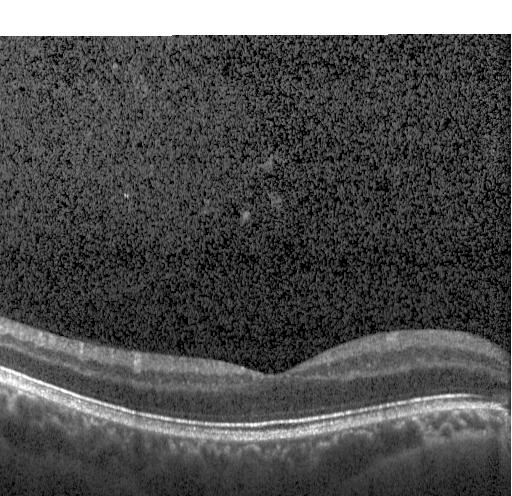 Retinal OCT cross-section showing no evidence of choroidal neovascularization, diabetic macular edema, or drusen.